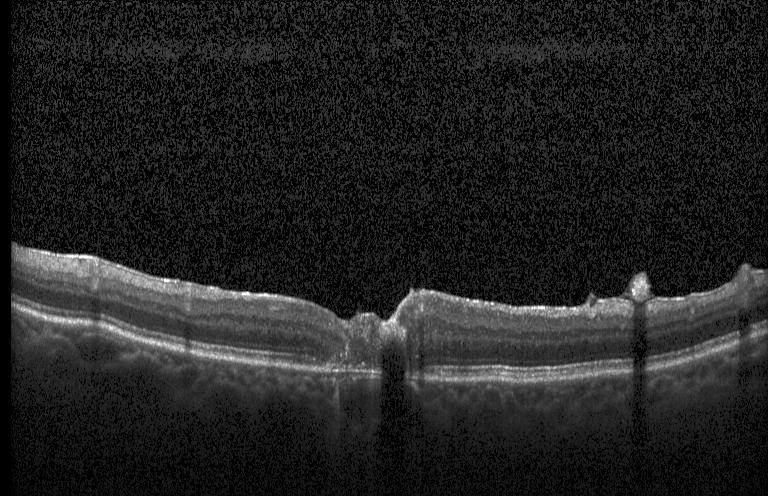 SD-OCT, retinal OCT B-scan
OCT finding: a choroidal neovascular membrane.